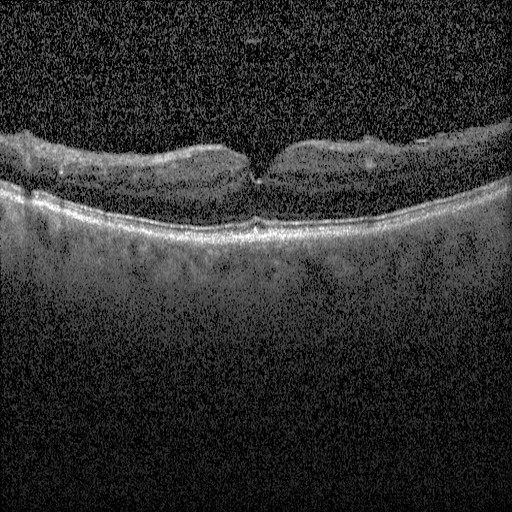
Retinal OCT B-scan — Diabetic macular edema.